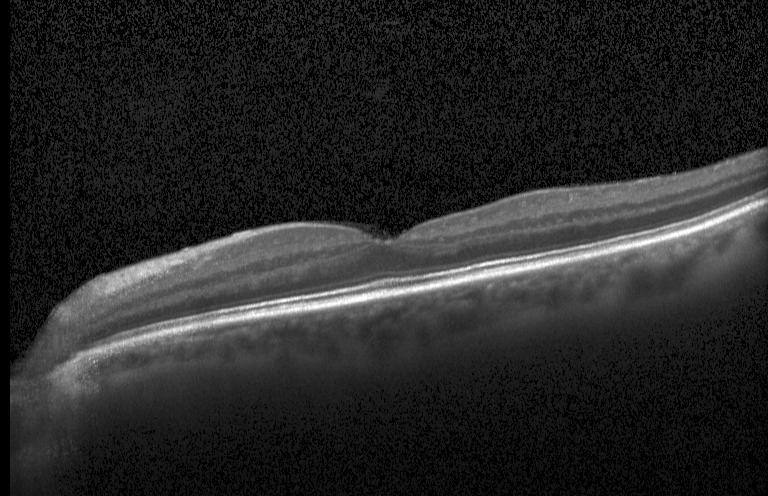

Spectral-domain OCT · acquired on a Heidelberg Spectralis · OCT B-scan.
Macular OCT: no choroidal neovascularization, no diabetic macular edema, and no drusen.